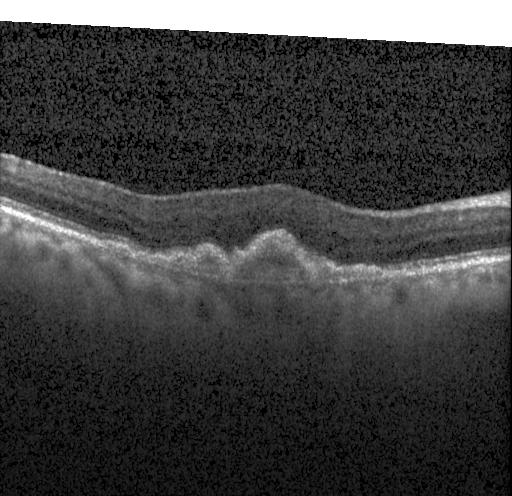
Impression: choroidal neovascularization (CNV).